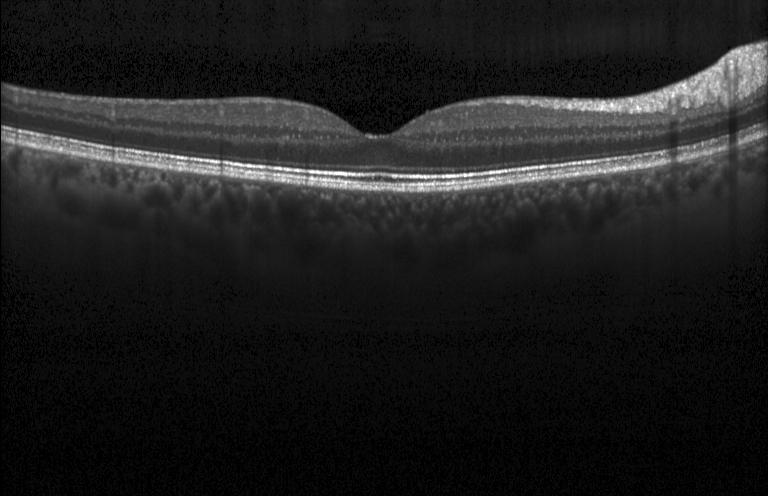

Assessment: no choroidal neovascularization, no diabetic macular edema, and no drusen.